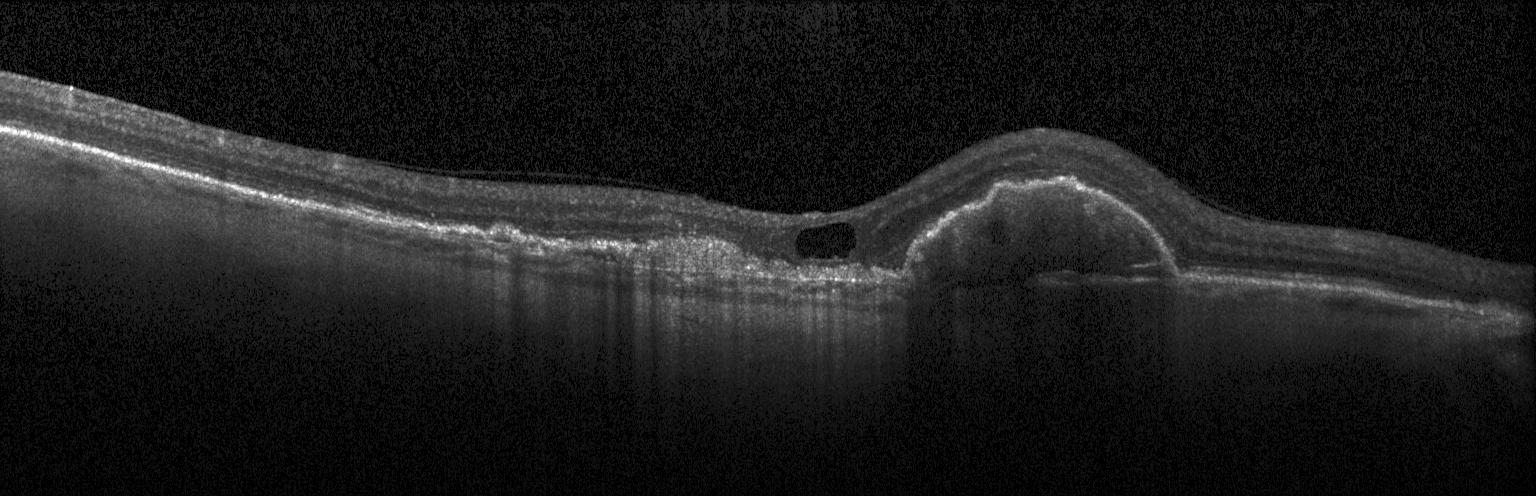

Retinal OCT cross-section · macular scan · Heidelberg Spectralis OCT system. Impression: choroidal neovascularization.